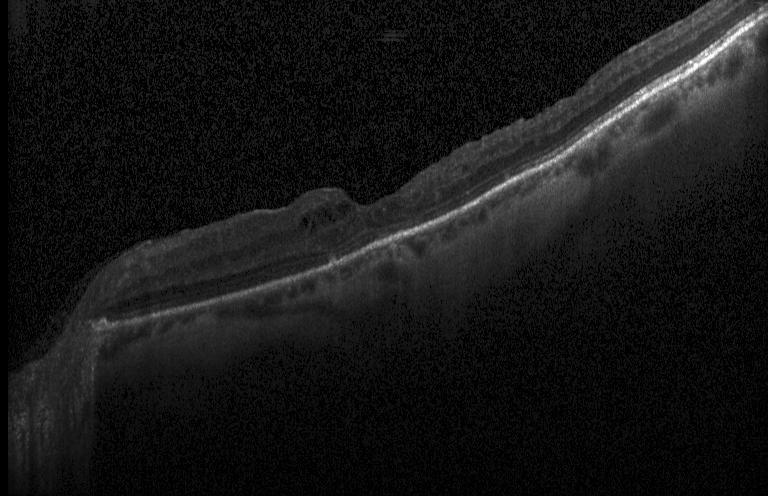 OCT B-scan; through the macula; SD-OCT.
OCT finding: diabetic macular edema (DME).